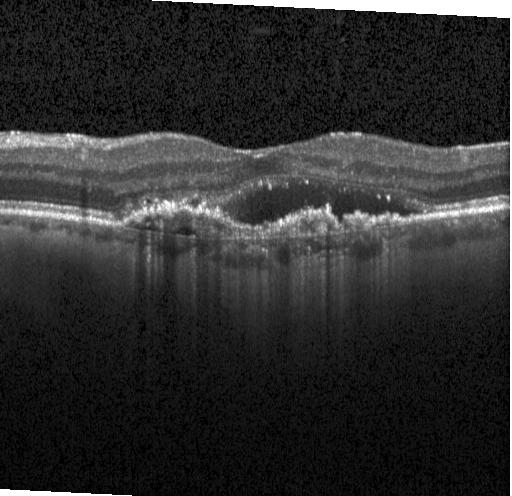 Retinal OCT B-scan. SD-OCT. Horizontal scan through the fovea
Finding: choroidal neovascularization.